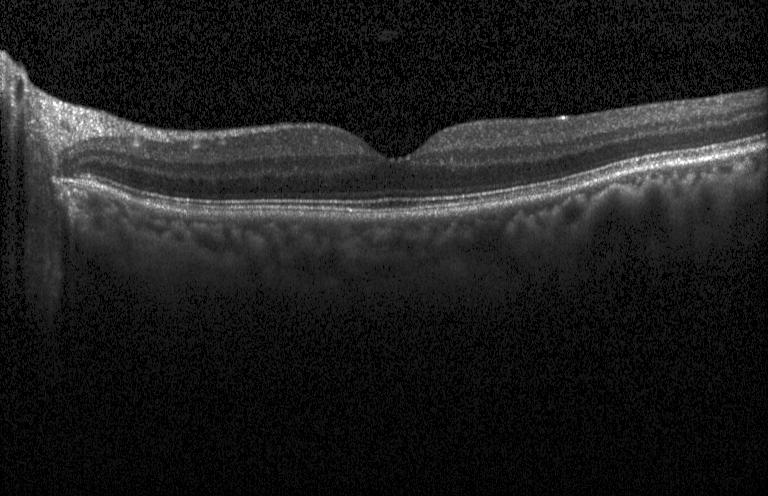 Spectral-domain OCT B-scan: no choroidal neovascularization, diabetic macular edema, or drusen.